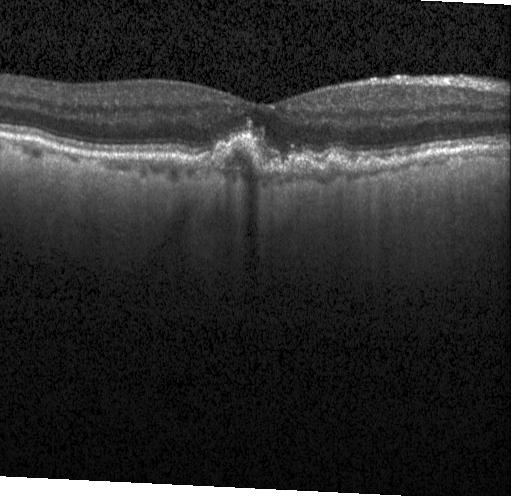

Acquired on a Heidelberg Spectralis. Spectral-domain OCT. Retinal OCT cross-section
Diagnosis: drusen.